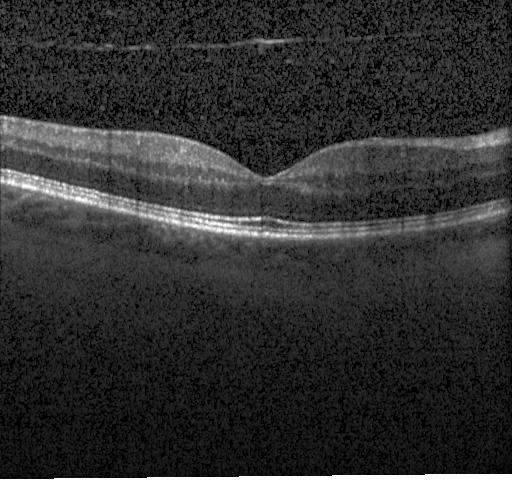 Retinal OCT cross-section showing neither choroidal neovascularization, diabetic macular edema, nor drusen.